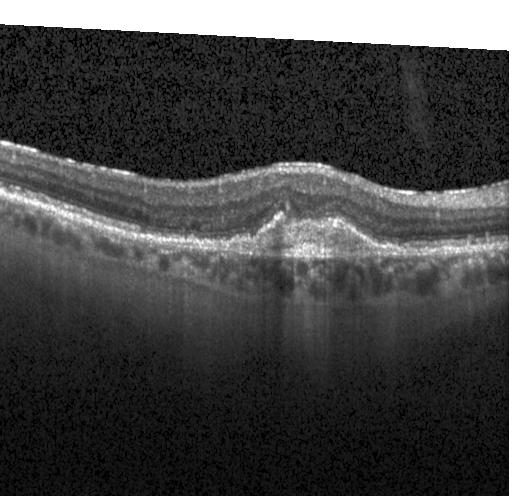

Macular OCT: CNV.